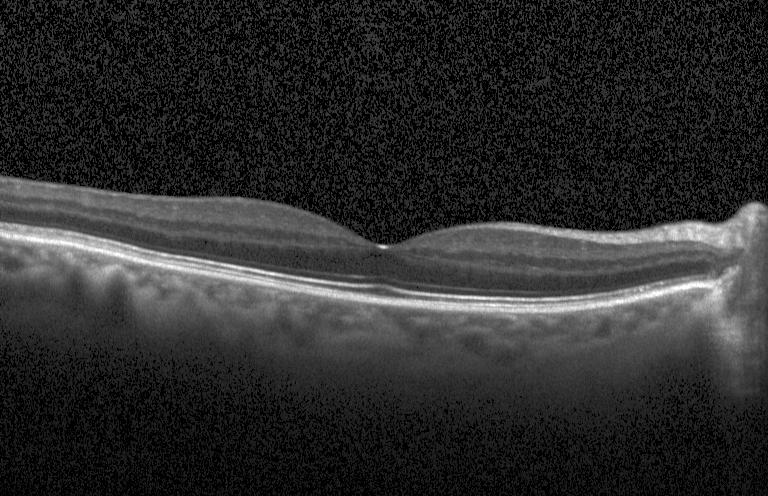 OCT B-scan · centered on the fovea · spectral-domain OCT
Neither CNV, DME, nor drusen.